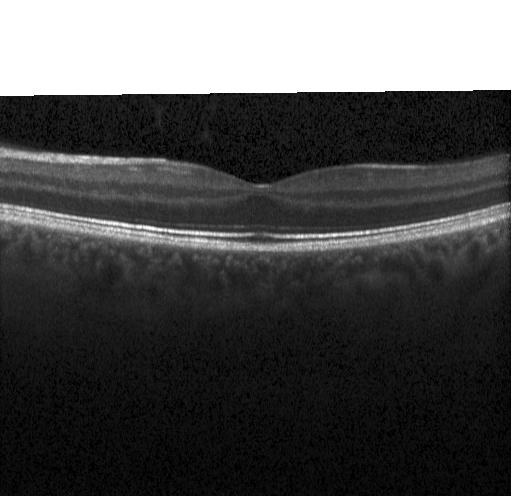
Impression: neither CNV, DME, nor drusen.